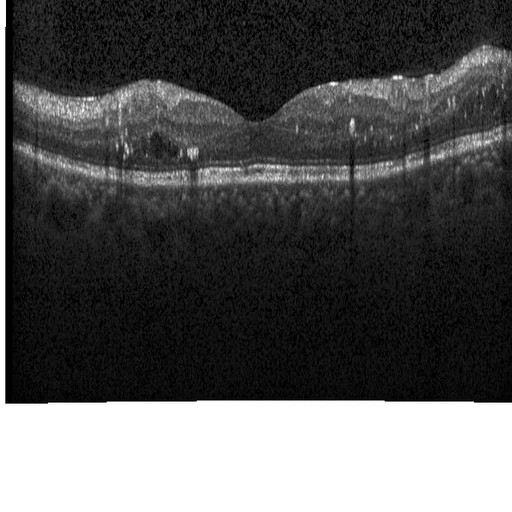 This B-scan demonstrates diabetic macular edema.